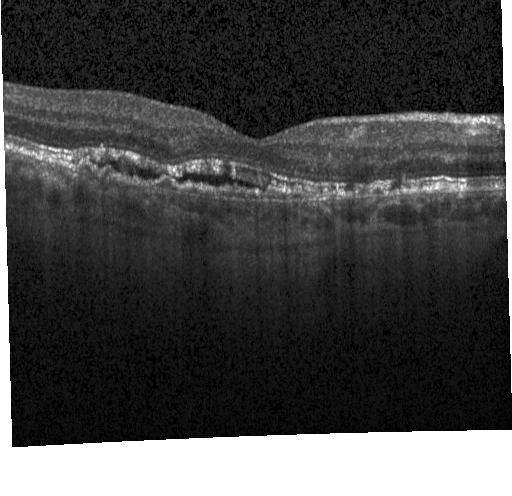

Finding: choroidal neovascularization.